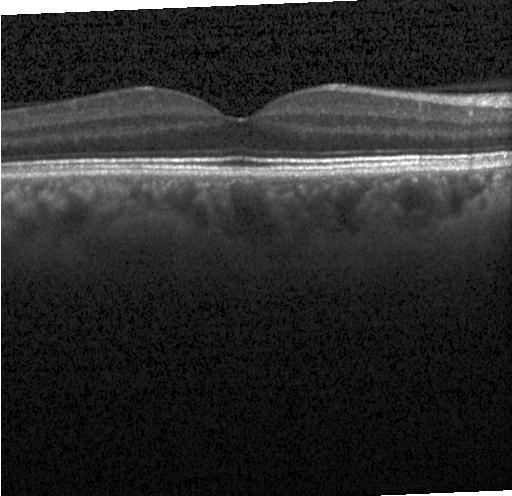
OCT B-scan. Heidelberg Spectralis. Fovea-centered.
This B-scan demonstrates no CNV, no DME, and no drusen.